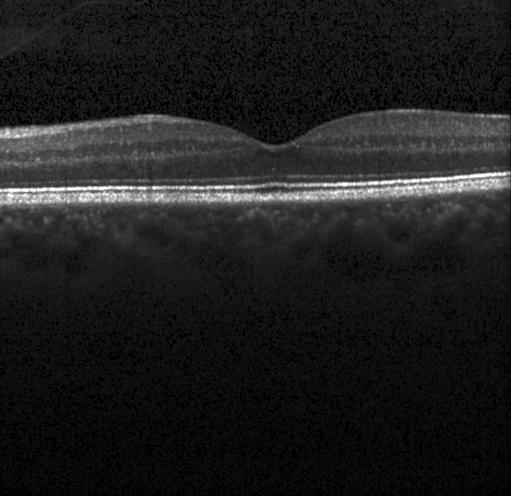
Optical coherence tomography scan. Finding: no evidence of choroidal neovascularization, diabetic macular edema, or drusen.